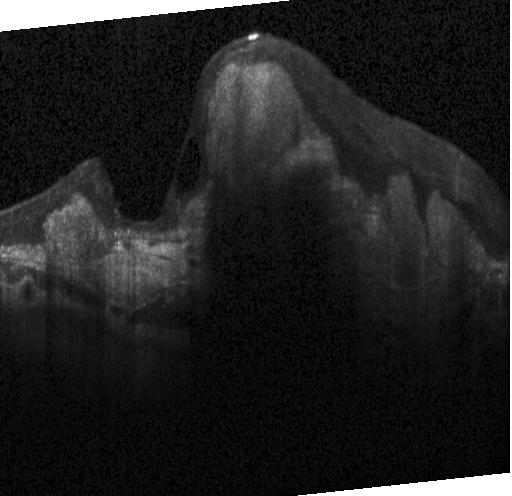
Diagnosis: choroidal neovascularization.